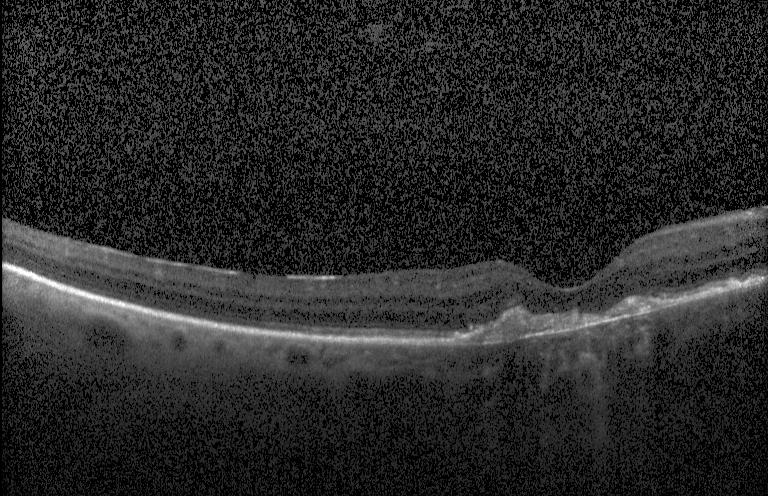
Retinal OCT cross-section. Through the macula. Instrument: Heidelberg Spectralis.
This B-scan demonstrates a choroidal neovascular membrane.